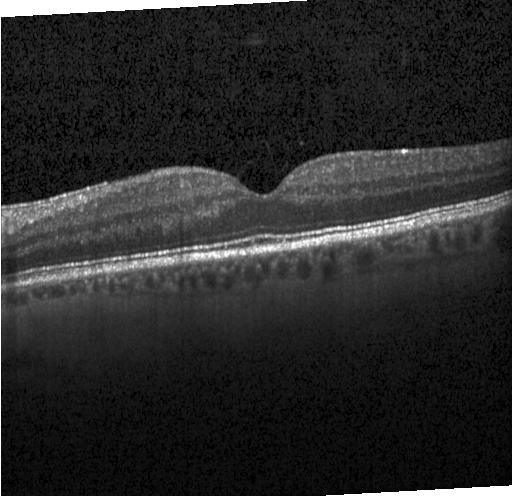

Dx: neither choroidal neovascularization, diabetic macular edema, nor drusen.